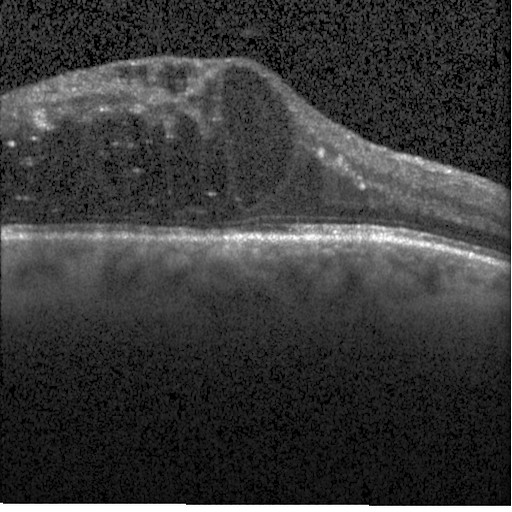

OCT finding: diabetic macular edema (DME).